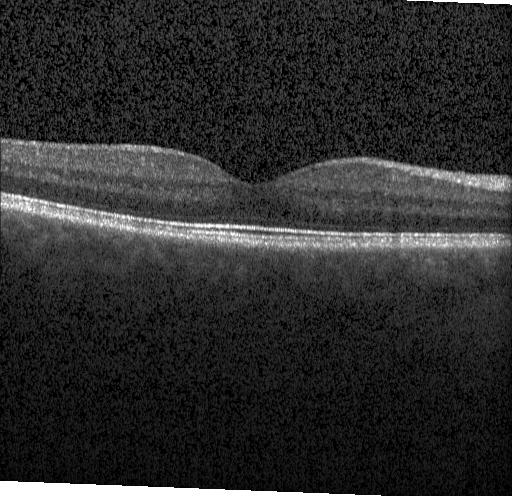
Diagnosis: neither choroidal neovascularization, diabetic macular edema, nor drusen.